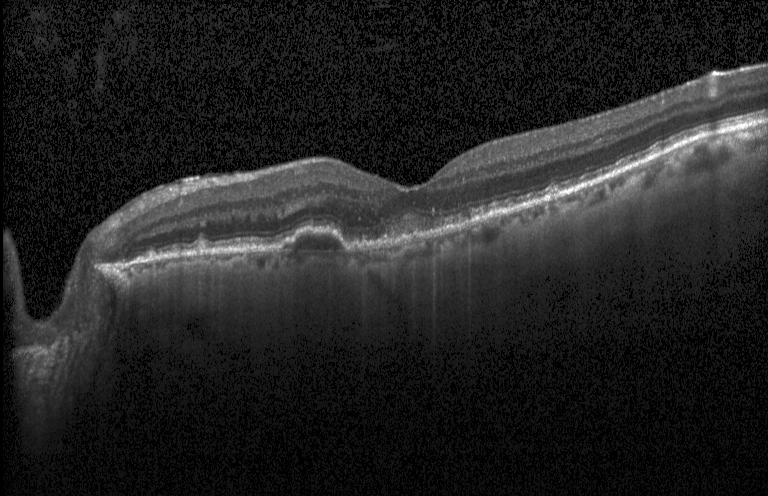 OCT B-scan showing choroidal neovascularization.